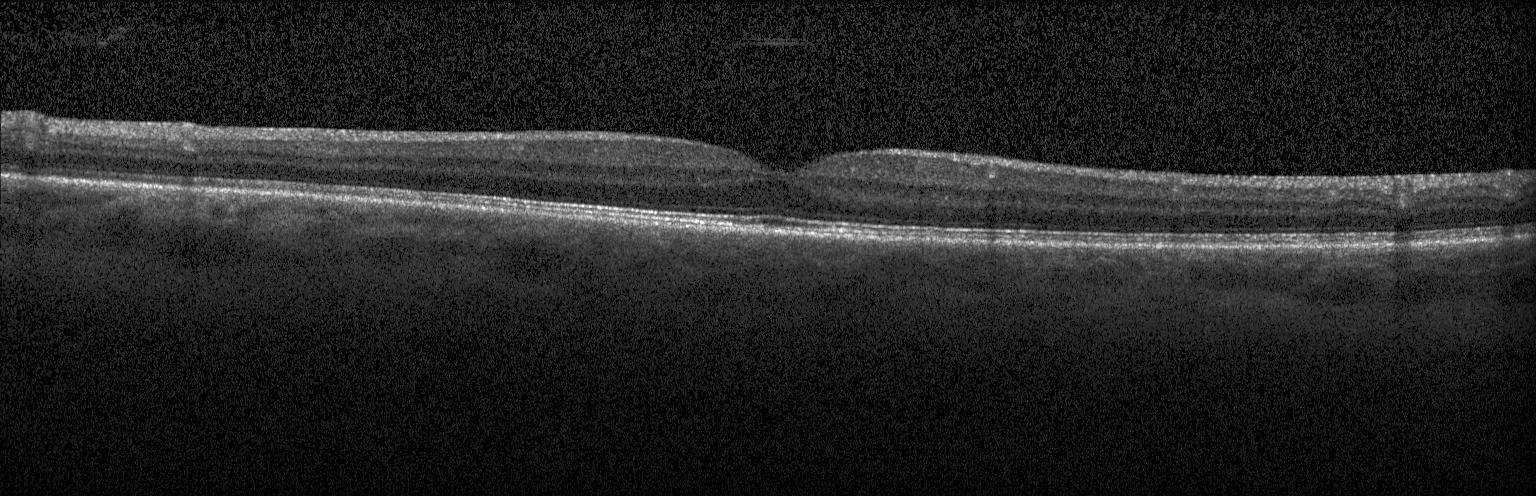
Optical coherence tomography scan
Assessment: no evidence of choroidal neovascularization, diabetic macular edema, or drusen.